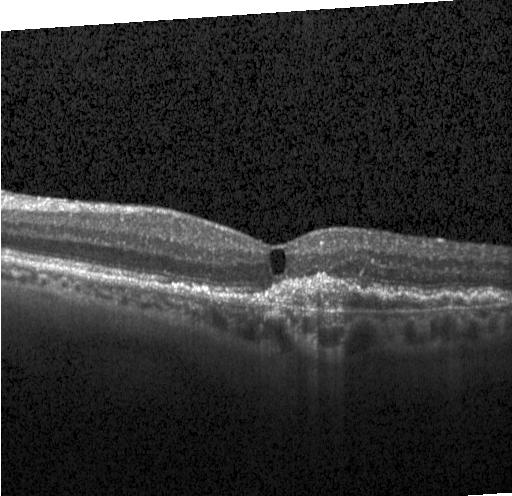

Spectral-domain OCT B-scan: choroidal neovascularization (CNV).